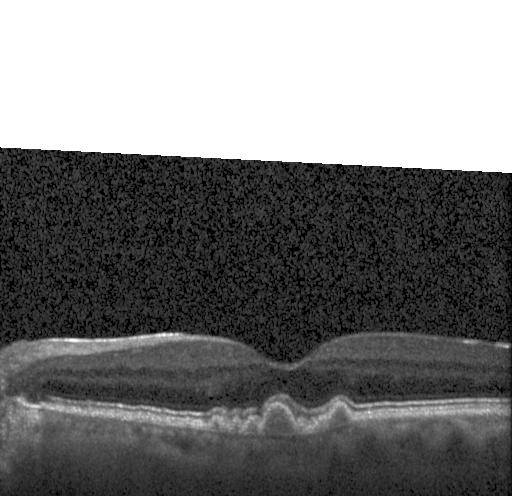

Diagnosis: multiple drusen.